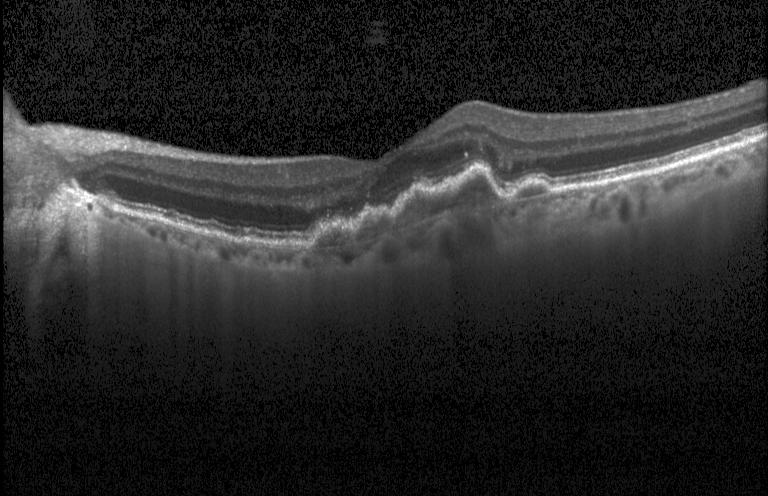
Spectral-domain OCT; Heidelberg Spectralis OCT system; centered on the fovea; retinal OCT B-scan — Finding: a choroidal neovascular membrane.